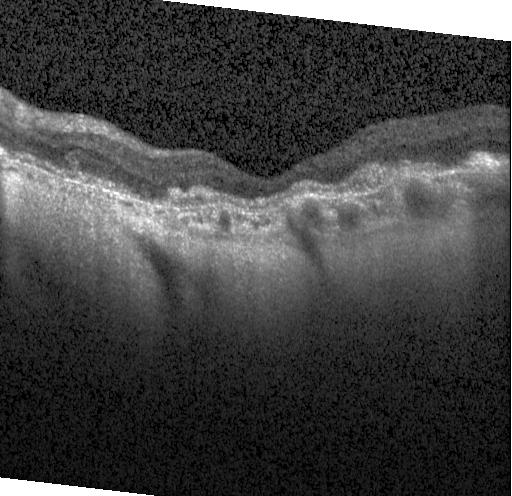 OCT scan showing a choroidal neovascular membrane.